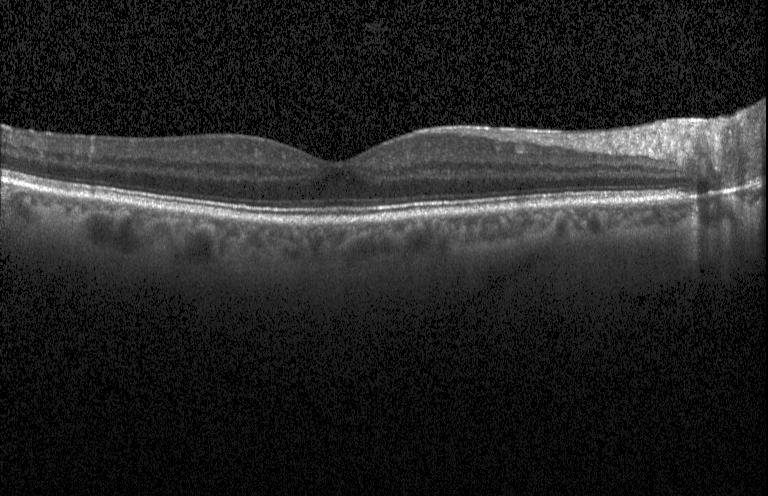 Fovea-centered · instrument: Heidelberg Spectralis · OCT line scan
The scan shows no choroidal neovascularization, no diabetic macular edema, and no drusen.